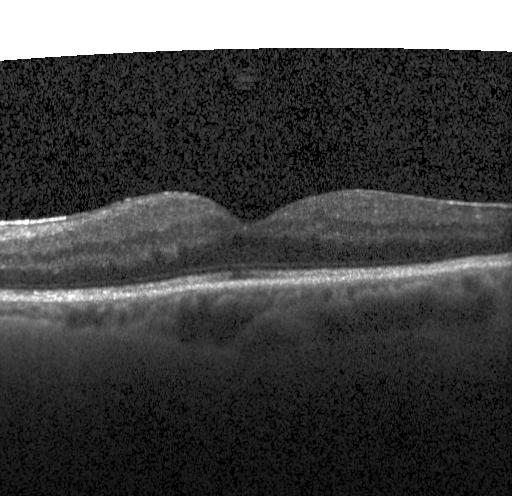 Acquired on a Heidelberg Spectralis, fovea-centered, retinal OCT cross-section, spectral-domain optical coherence tomography
The scan shows no evidence of choroidal neovascularization, diabetic macular edema, or drusen.